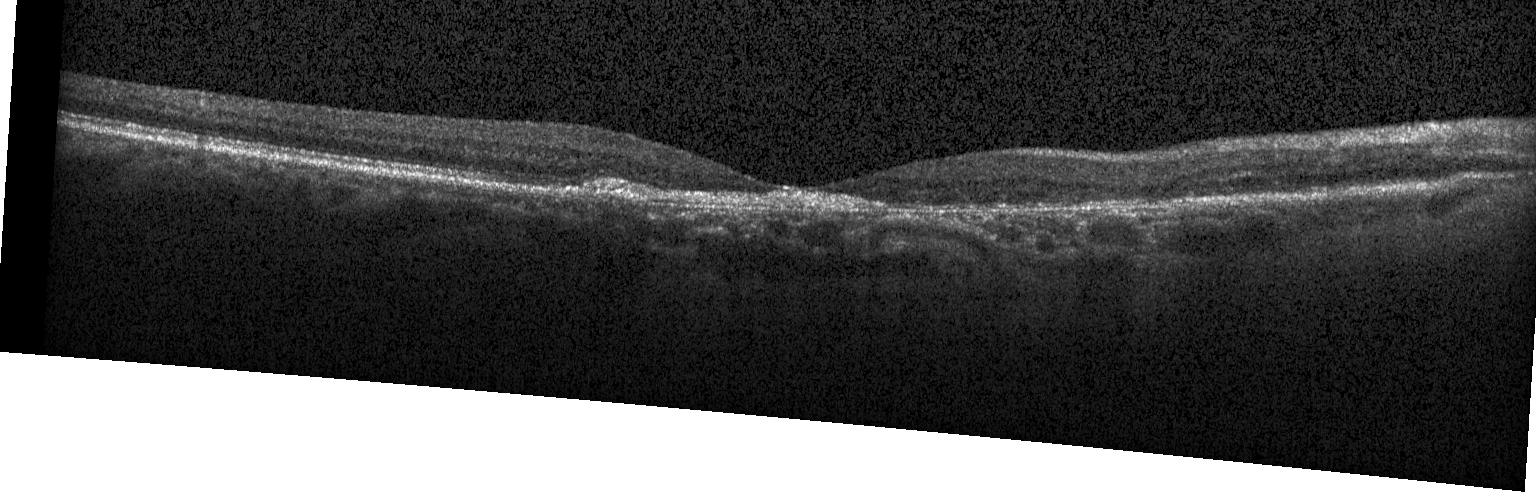 Through the macula. OCT line scan — The scan shows CNV.